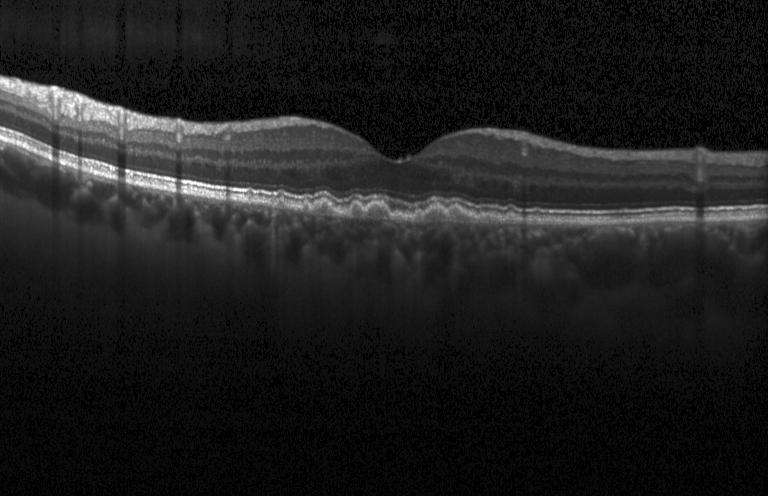

Impression: drusen.